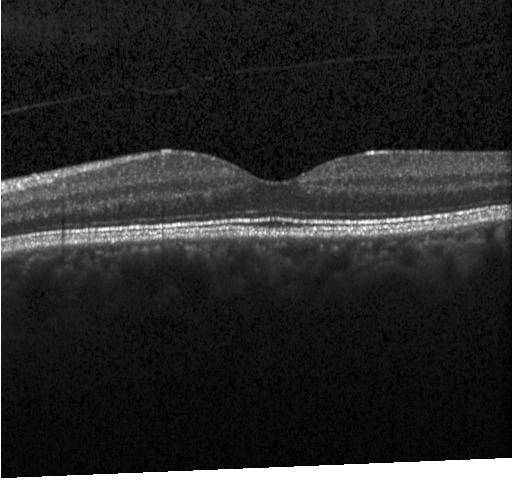

OCT line scan
This B-scan demonstrates no evidence of CNV, DME, or drusen.